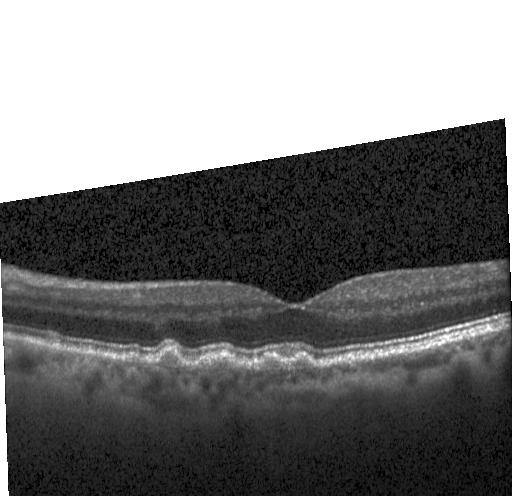 SD-OCT; fovea-centered; OCT line scan — Drusen.